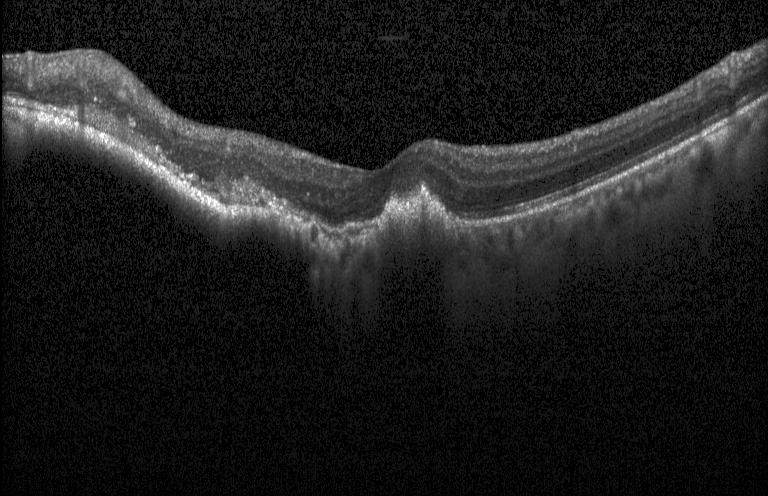 Macular OCT: a choroidal neovascular membrane.